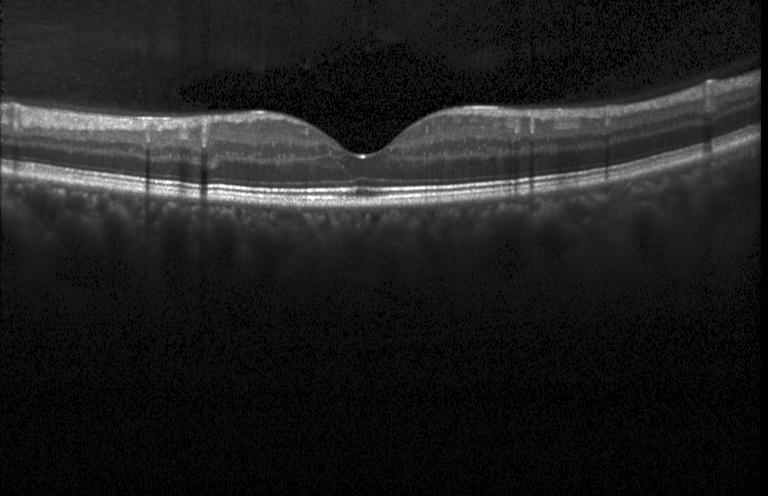 OCT B-scan showing neither choroidal neovascularization, diabetic macular edema, nor drusen.